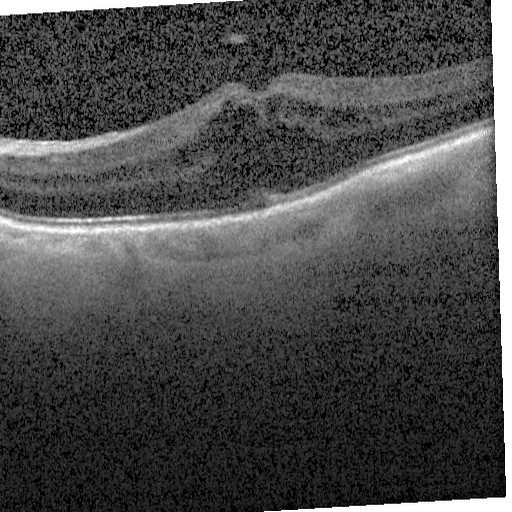 Instrument: Heidelberg Spectralis; horizontal scan through the fovea; optical coherence tomography scan; SD-OCT — Diagnosis: diabetic macular edema.